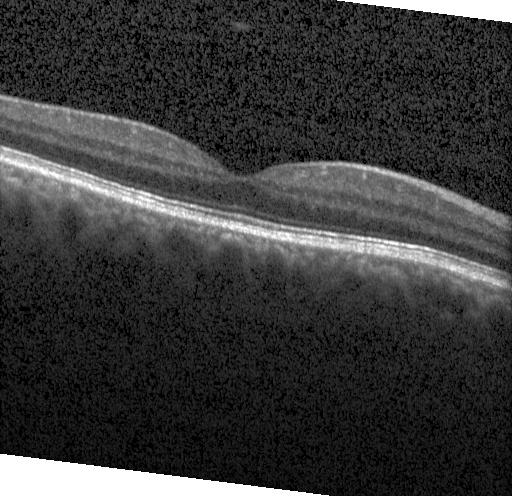 Assessment: neither choroidal neovascularization, diabetic macular edema, nor drusen.